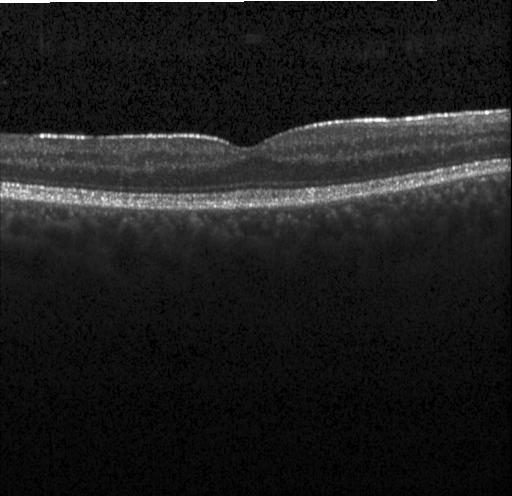 Finding: no CNV, no DME, and no drusen.